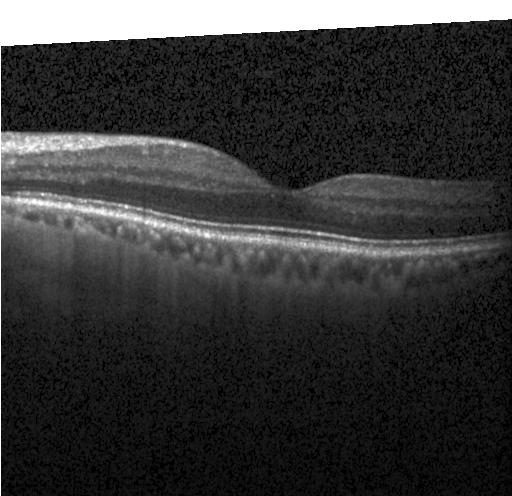
This B-scan demonstrates no choroidal neovascularization, no diabetic macular edema, and no drusen.